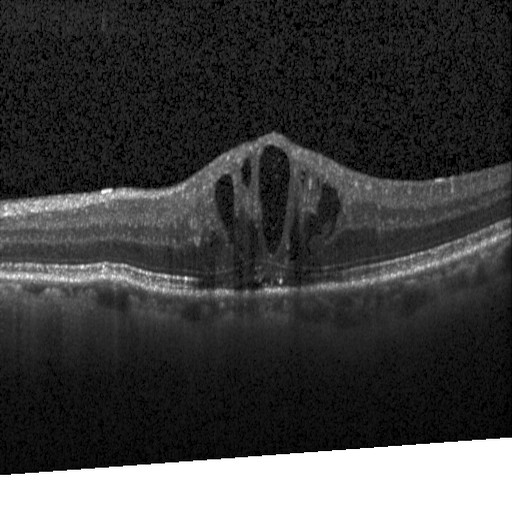 Centered on the fovea · optical coherence tomography B-scan. Impression: diabetic macular edema.